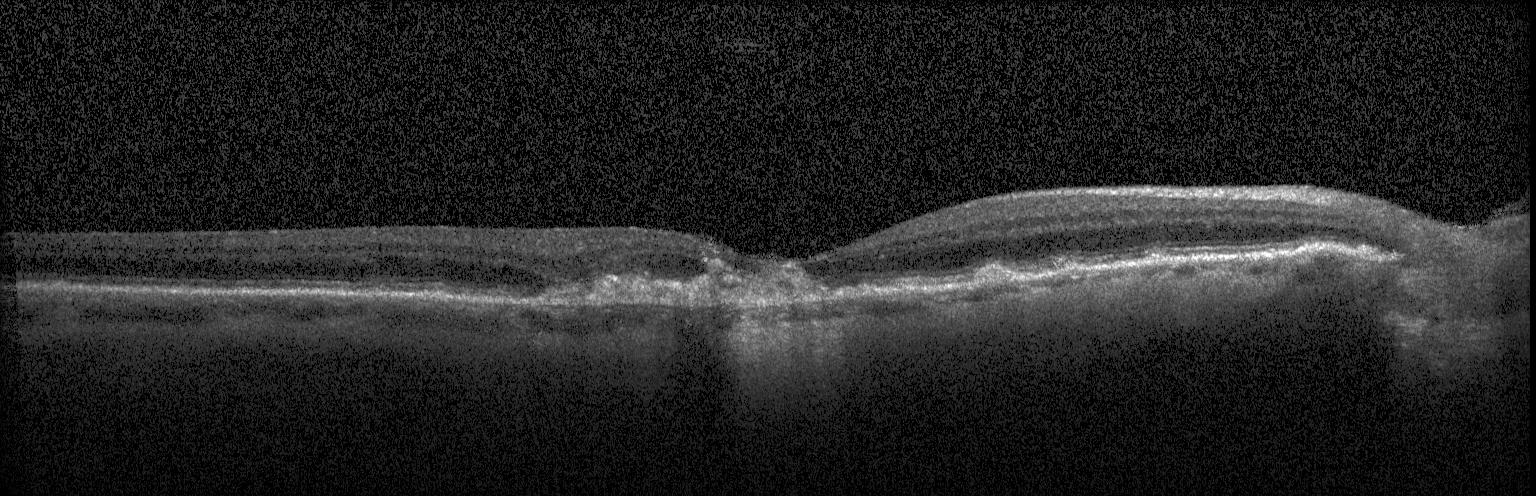

Choroidal neovascularization (CNV).